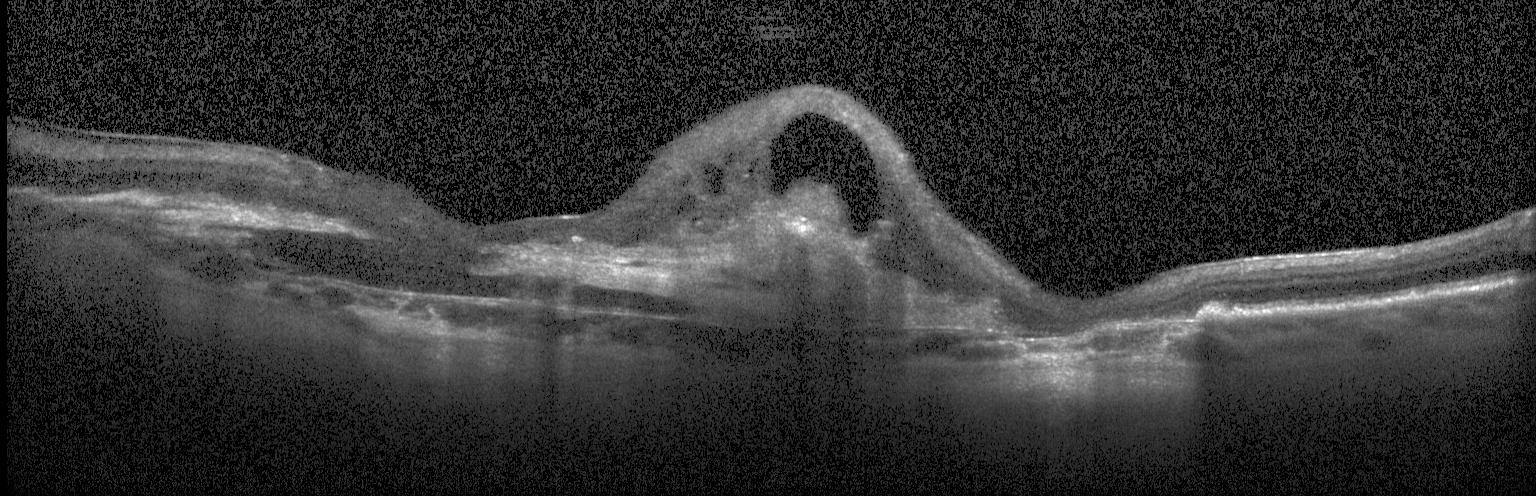

OCT B-scan. Impression: a choroidal neovascular membrane.